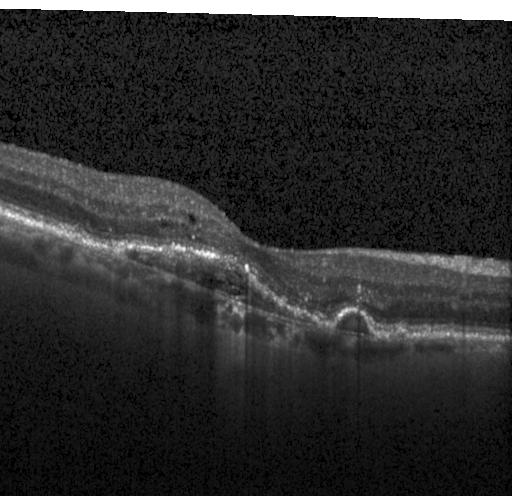

Retinal OCT B-scan; fovea-centered; spectral-domain OCT. OCT finding: choroidal neovascularization.